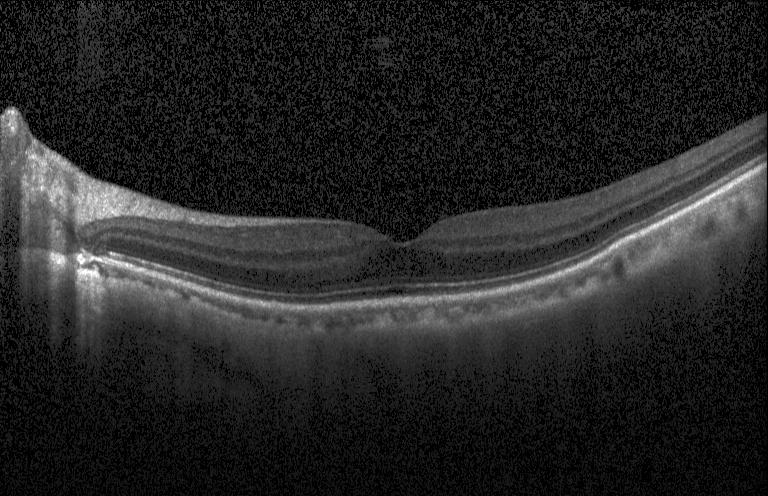

Horizontal scan through the fovea, optical coherence tomography scan.
Diagnosis: no evidence of choroidal neovascularization, diabetic macular edema, or drusen.